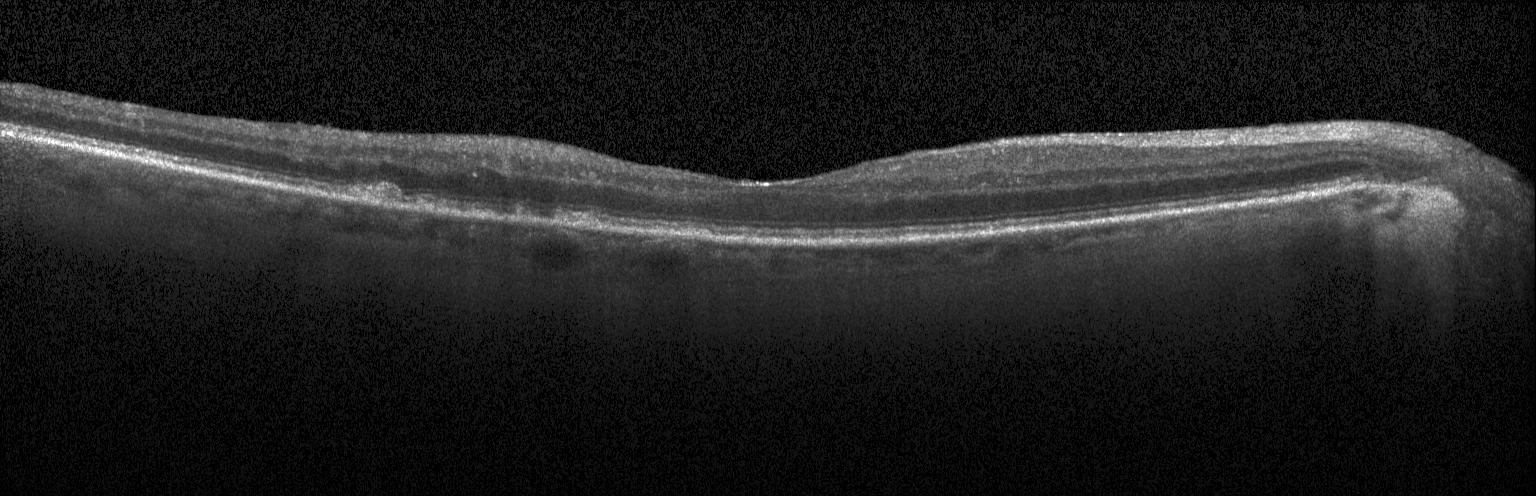 Retinal OCT B-scan; centered on the fovea. OCT finding: multiple drusen.